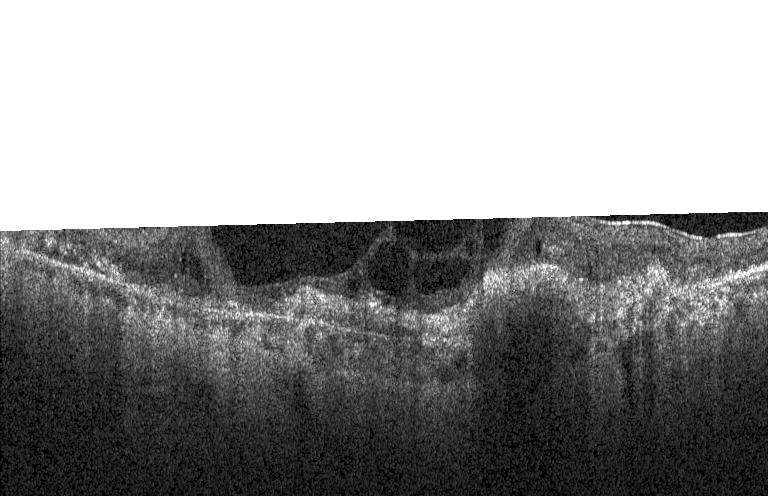 Macular OCT: a choroidal neovascular membrane.